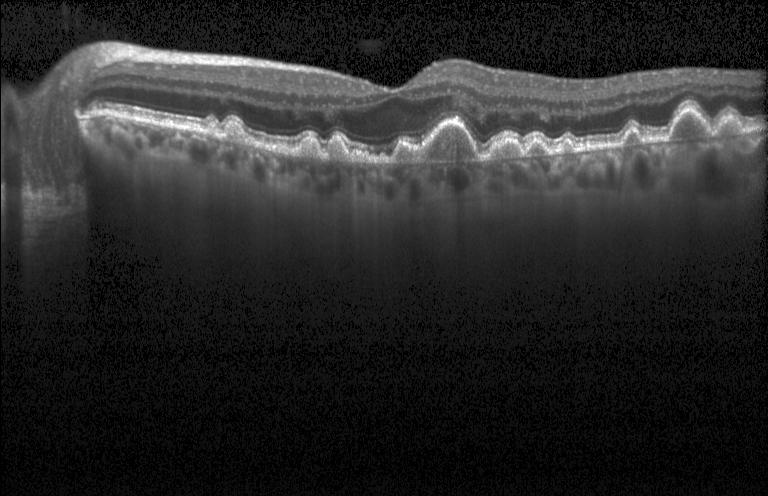 Heidelberg Spectralis OCT system. Retinal OCT cross-section. Spectral-domain OCT. Finding: multiple drusen.